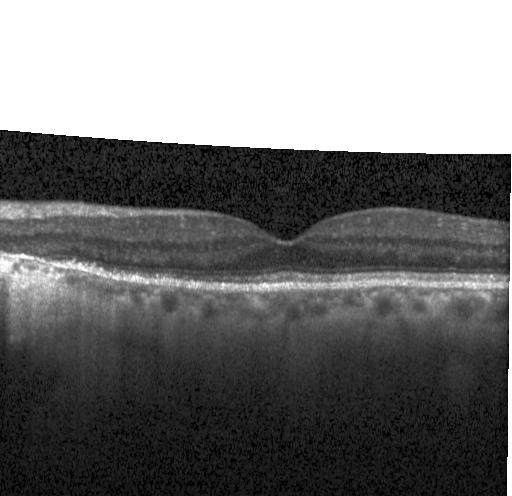
Retinal OCT cross-section. Fovea-centered. Heidelberg Spectralis.
Diagnosis: no choroidal neovascularization, diabetic macular edema, or drusen.